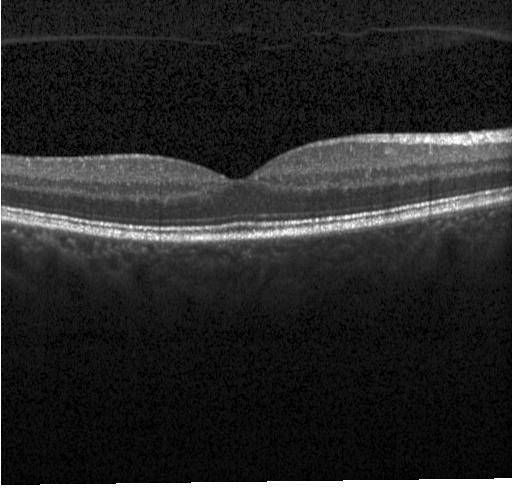

SD-OCT. Retinal OCT cross-section. Fovea-centered.
Diagnosis: neither CNV, DME, nor drusen.